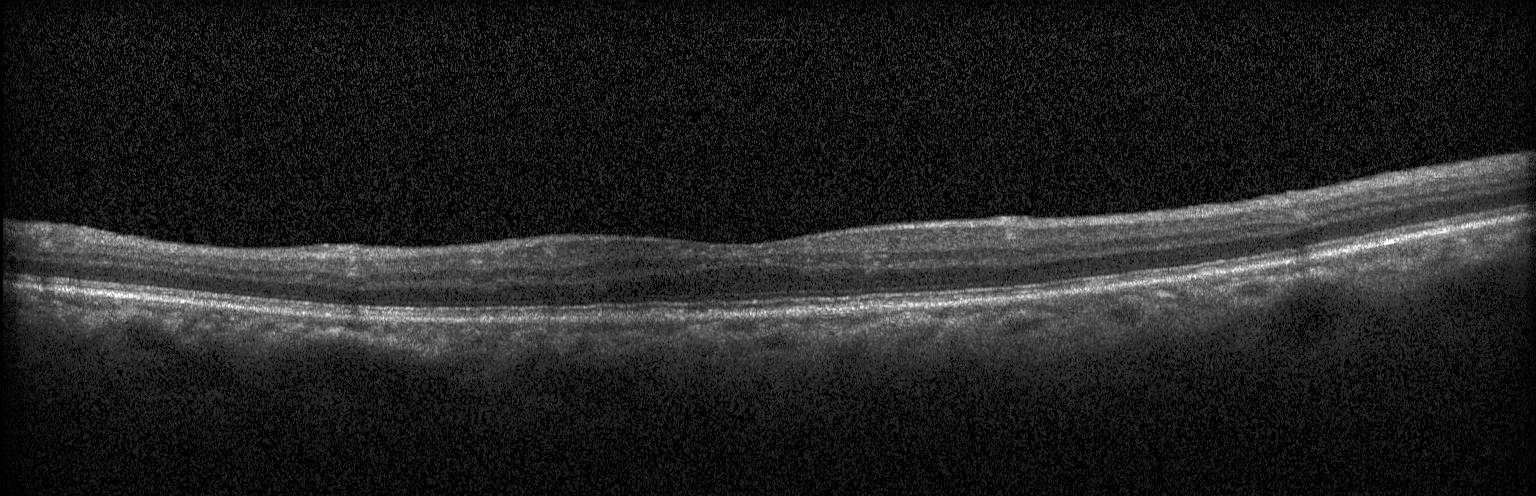 Optical coherence tomography scan; horizontal scan through the fovea; Heidelberg Spectralis OCT system; SD-OCT — Finding: neither CNV, DME, nor drusen.